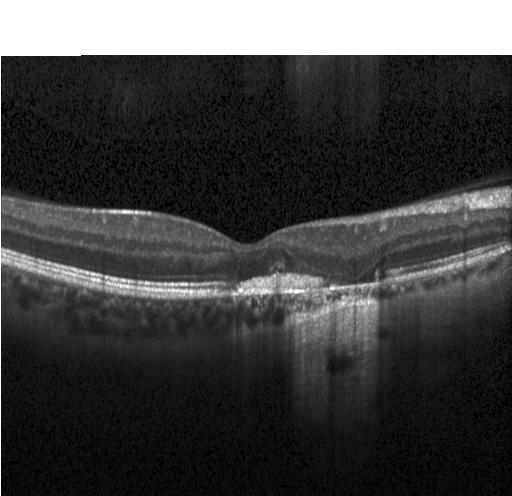

OCT B-scan showing a choroidal neovascular membrane.